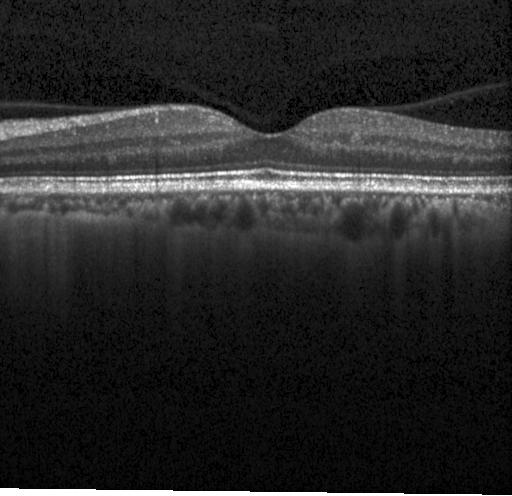 Optical coherence tomography B-scan, acquired on a Heidelberg Spectralis, SD-OCT, through the macula
Dx: neither choroidal neovascularization, diabetic macular edema, nor drusen.